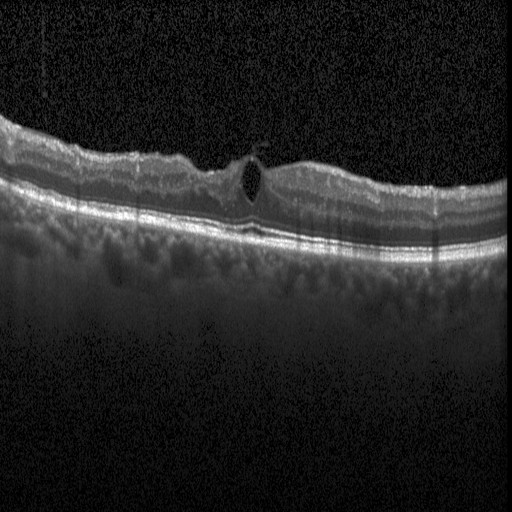
OCT B-scan
Impression: diabetic macular edema.